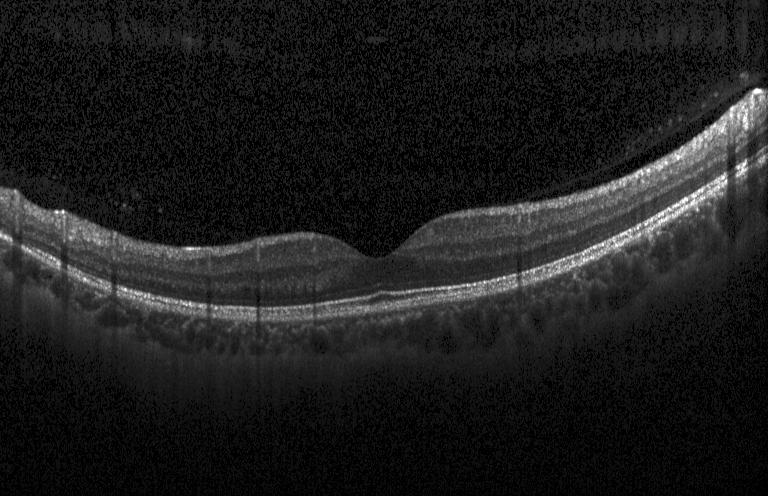
Assessment: no evidence of CNV, DME, or drusen.